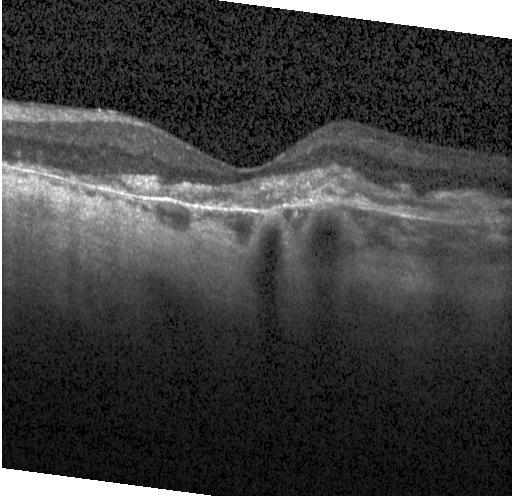
Spectral-domain OCT B-scan: choroidal neovascularization.